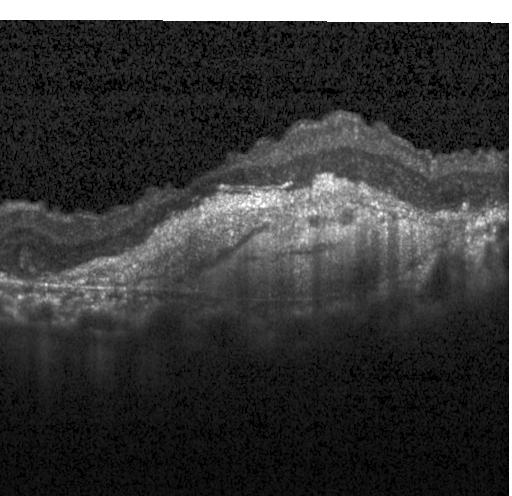

OCT B-scan
This B-scan demonstrates a choroidal neovascular membrane.